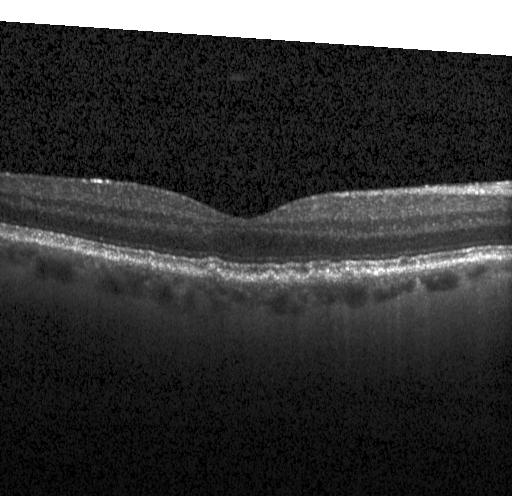 OCT B-scan. Diagnosis: multiple drusen.